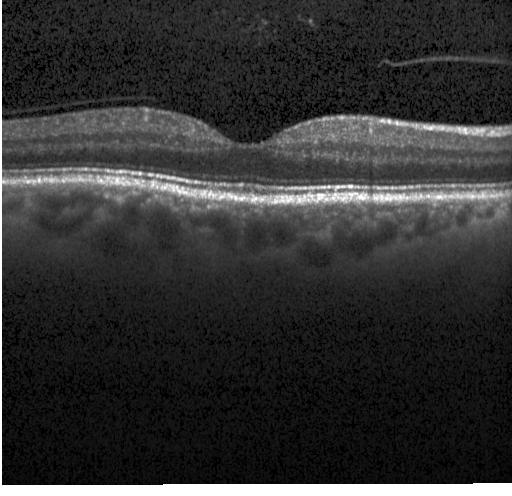
Spectral-domain optical coherence tomography · optical coherence tomography B-scan · acquired on a Heidelberg Spectralis · fovea-centered.
The scan shows neither choroidal neovascularization, diabetic macular edema, nor drusen.